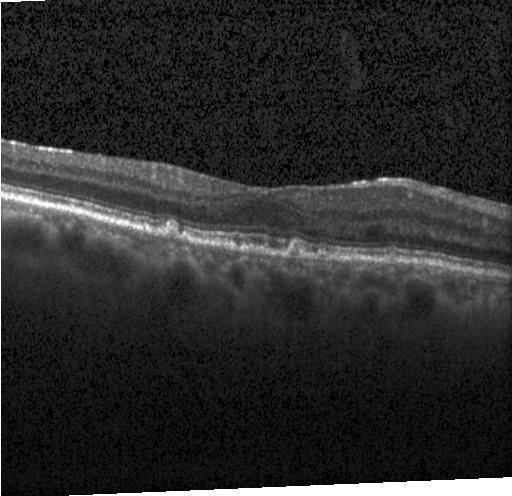
Finding: multiple drusen.